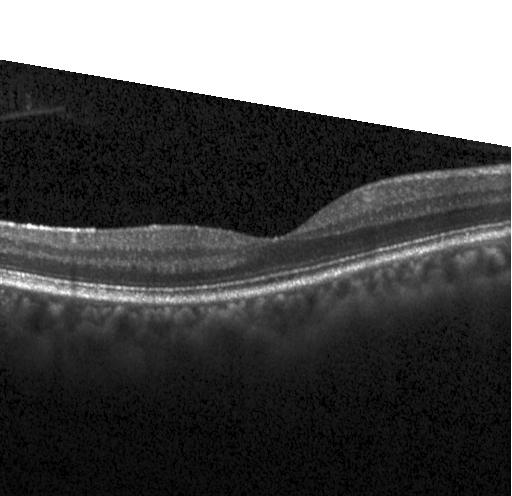

Optical coherence tomography scan, Heidelberg Spectralis
Macular OCT: no evidence of choroidal neovascularization, diabetic macular edema, or drusen.